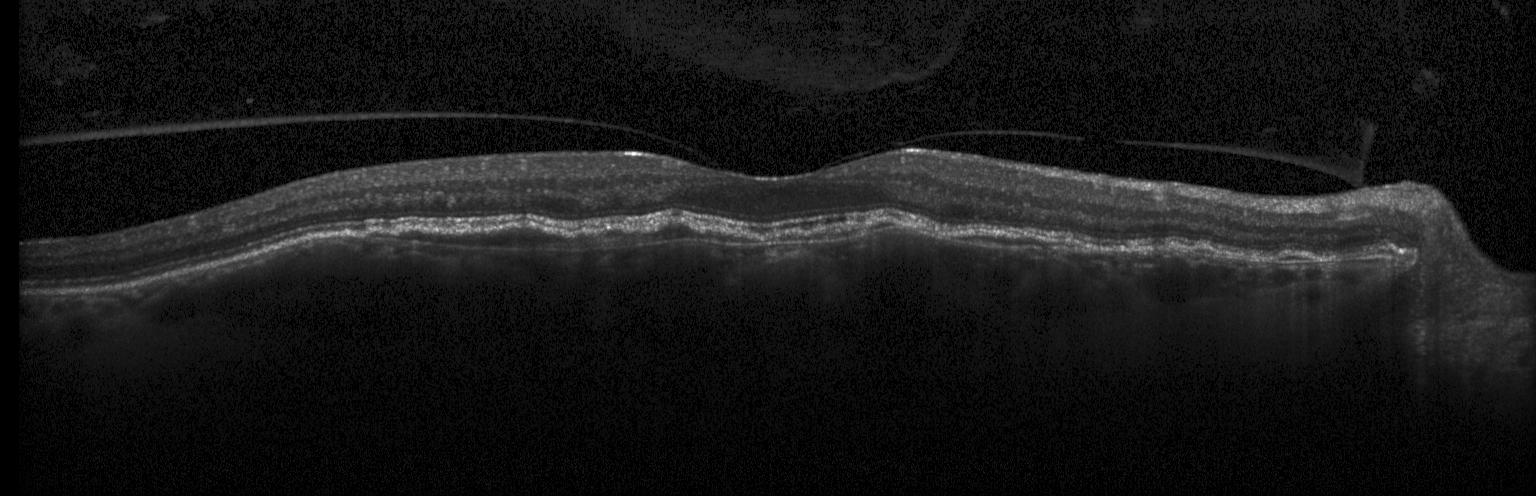
Acquired on a Heidelberg Spectralis; fovea-centered; SD-OCT; retinal OCT B-scan — Macular OCT: choroidal neovascularization.